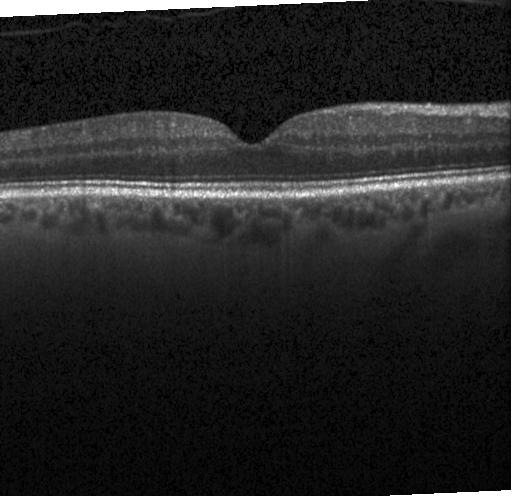 OCT line scan. Horizontal scan through the fovea. OCT finding: no evidence of choroidal neovascularization, diabetic macular edema, or drusen.